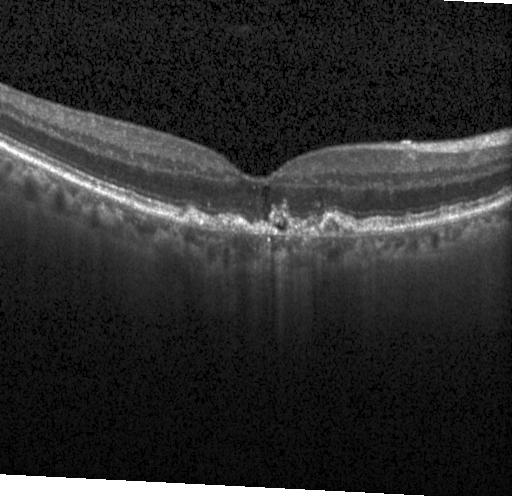 Horizontal scan through the fovea. Spectral-domain OCT. OCT B-scan. Heidelberg Spectralis — Diagnosis: choroidal neovascularization.